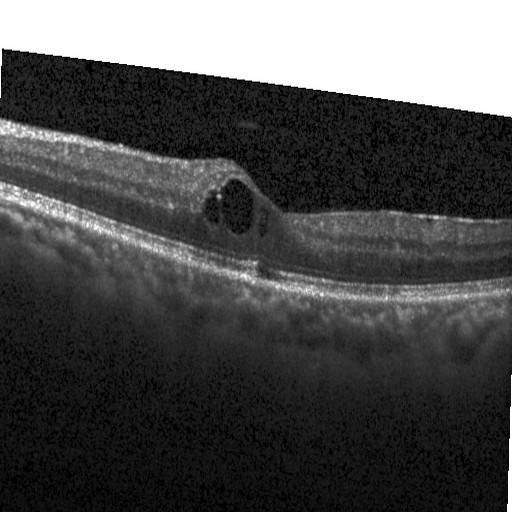 Heidelberg Spectralis OCT system, optical coherence tomography B-scan, spectral-domain OCT. The scan shows diabetic macular edema (DME).